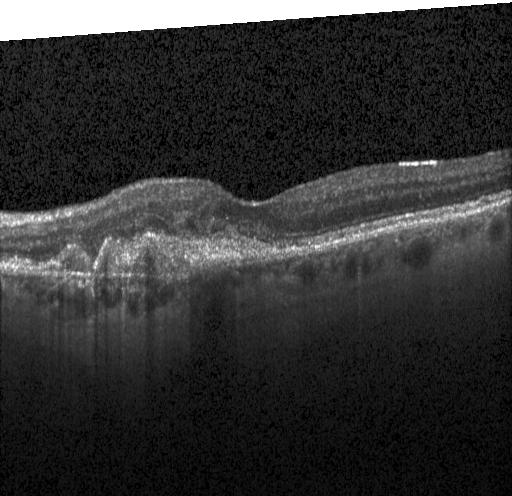

Finding: choroidal neovascularization.